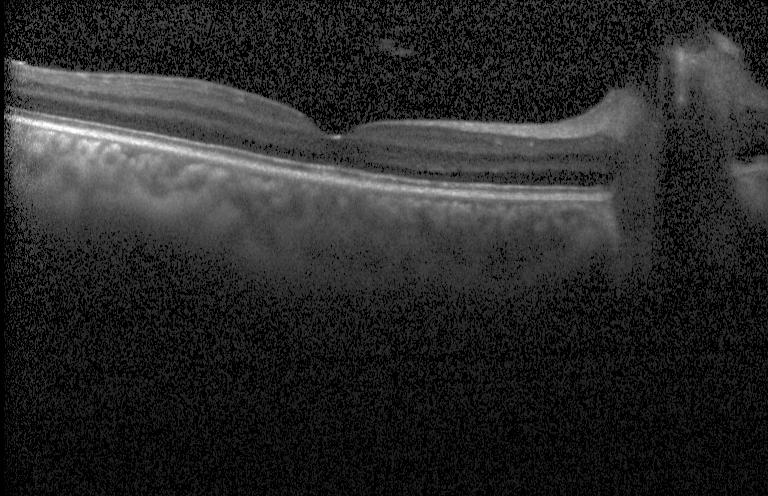

Retinal OCT cross-section showing neither choroidal neovascularization, diabetic macular edema, nor drusen.